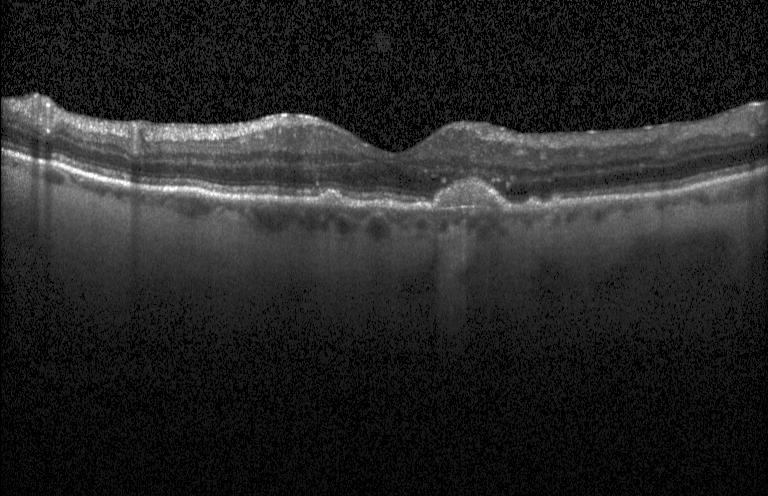
Fovea-centered · optical coherence tomography B-scan · acquired on a Heidelberg Spectralis
Assessment: a choroidal neovascular membrane.